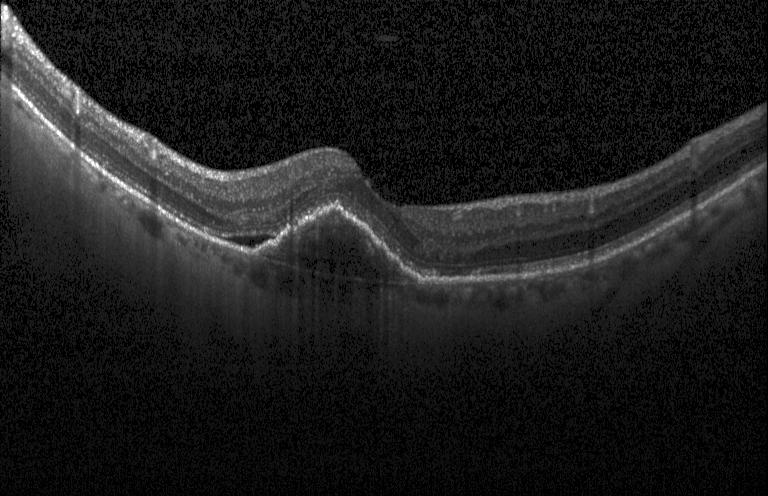

OCT line scan; acquired on a Heidelberg Spectralis; spectral-domain optical coherence tomography; macular scan — Assessment: choroidal neovascularization (CNV).